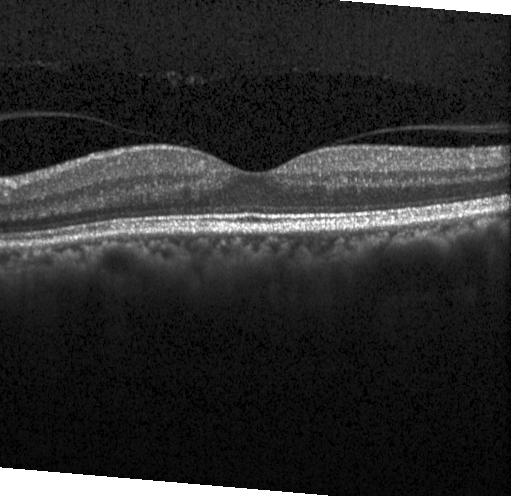 OCT line scan.
OCT finding: no choroidal neovascularization, diabetic macular edema, or drusen.